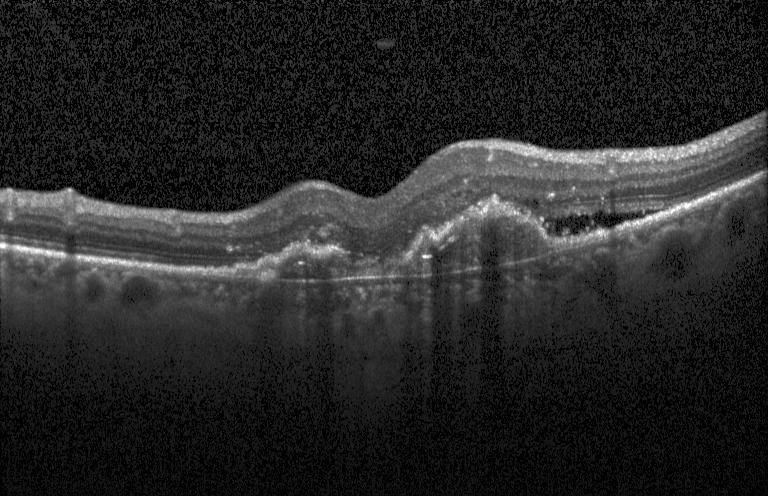
Macular OCT demonstrating a choroidal neovascular membrane.